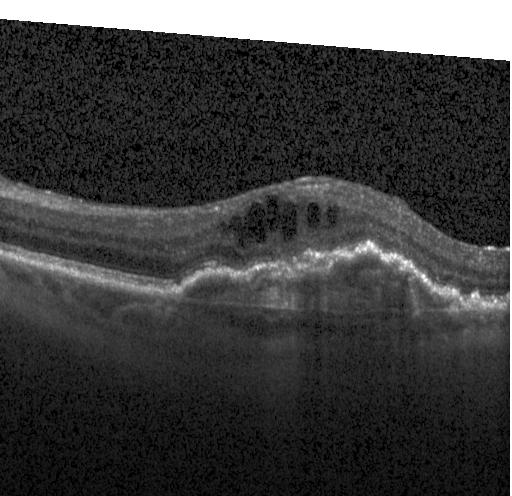

Impression: a choroidal neovascular membrane.